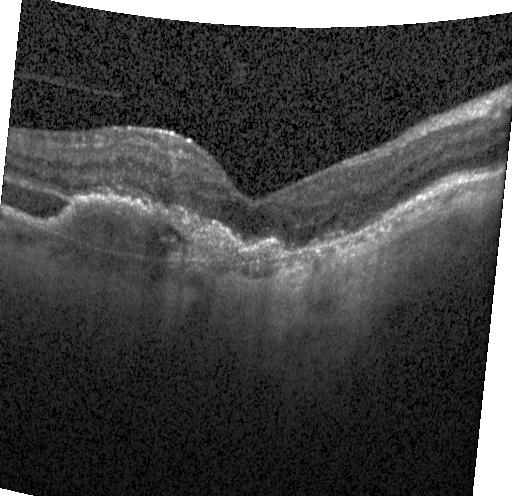
Impression: CNV.